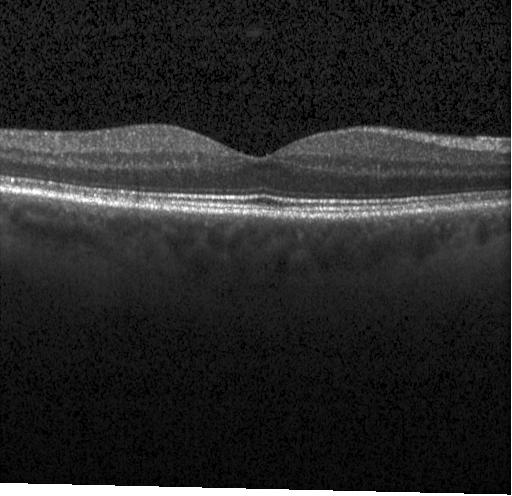 OCT line scan.
Diagnosis: no choroidal neovascularization, no diabetic macular edema, and no drusen.